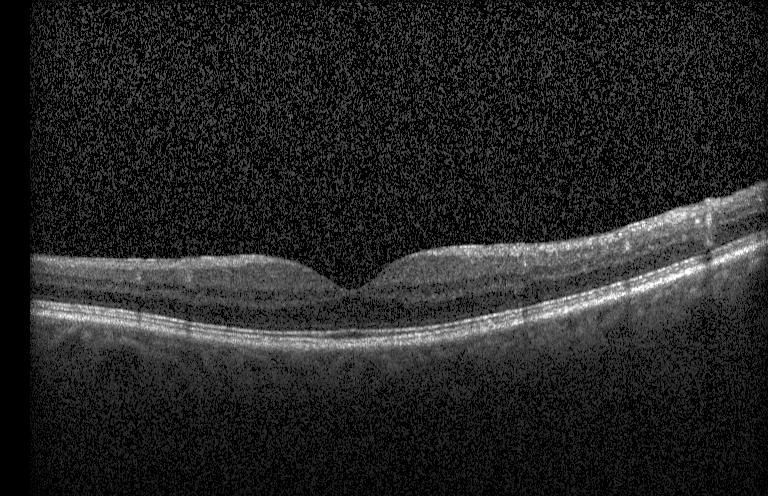 Optical coherence tomography B-scan.
Finding: neither CNV, DME, nor drusen.